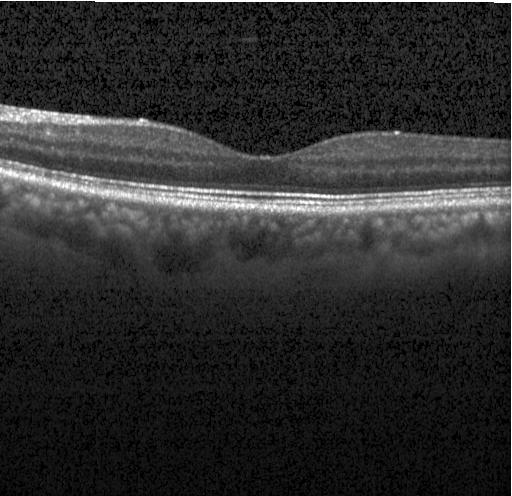
Spectral-domain OCT · acquired on a Heidelberg Spectralis · OCT line scan · through the macula. No CNV, no DME, and no drusen.